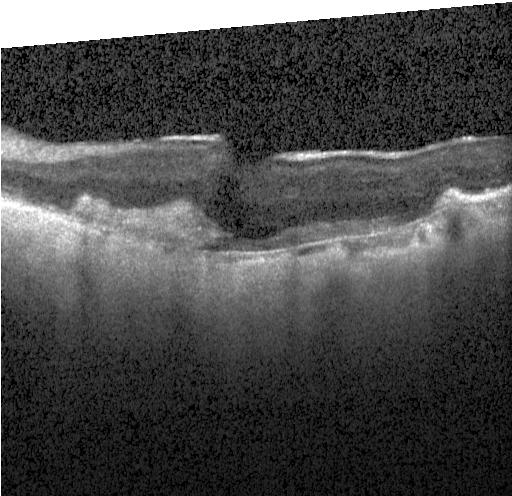

OCT line scan; SD-OCT; macular scan
Macular OCT: a choroidal neovascular membrane.